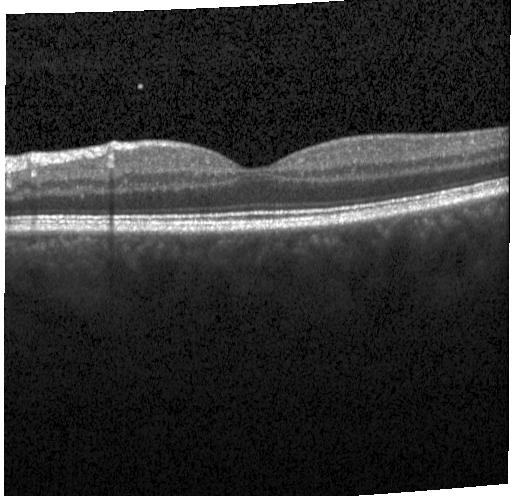

Optical coherence tomography B-scan — Diagnosis: neither choroidal neovascularization, diabetic macular edema, nor drusen.